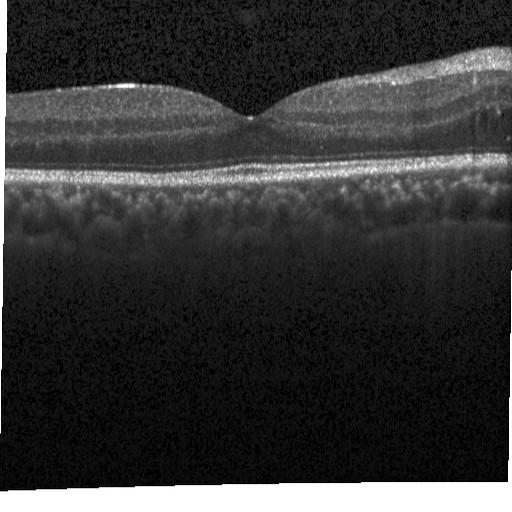

Macular OCT: DME.